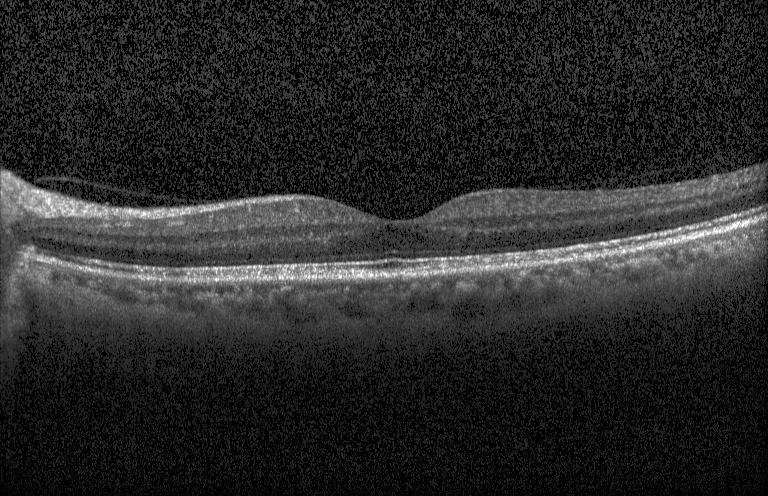 Optical coherence tomography scan
No evidence of CNV, DME, or drusen.